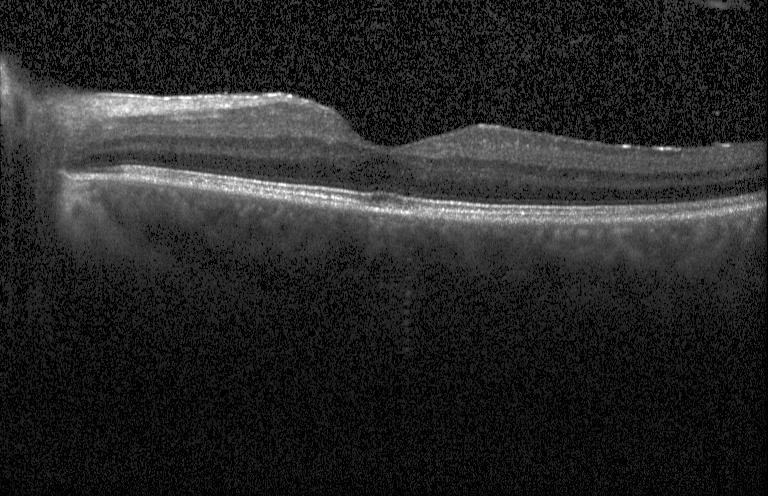
Spectral-domain optical coherence tomography; OCT B-scan
Finding: no evidence of choroidal neovascularization, diabetic macular edema, or drusen.